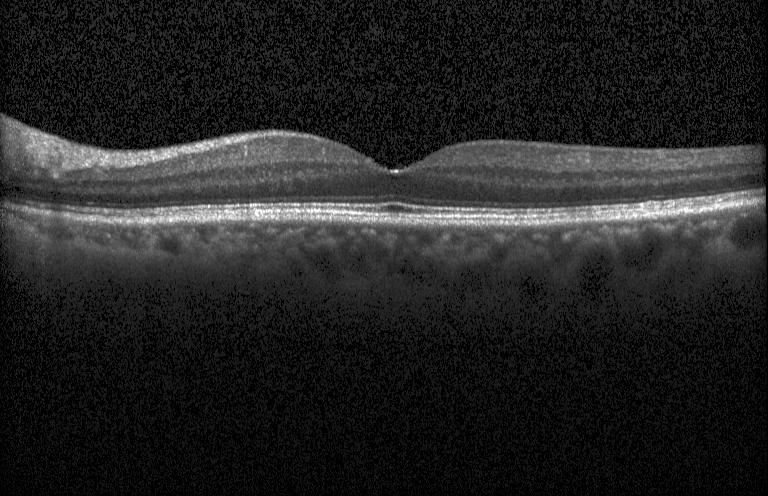 Heidelberg Spectralis, fovea-centered, OCT B-scan, spectral-domain optical coherence tomography
Finding: no choroidal neovascularization, diabetic macular edema, or drusen.